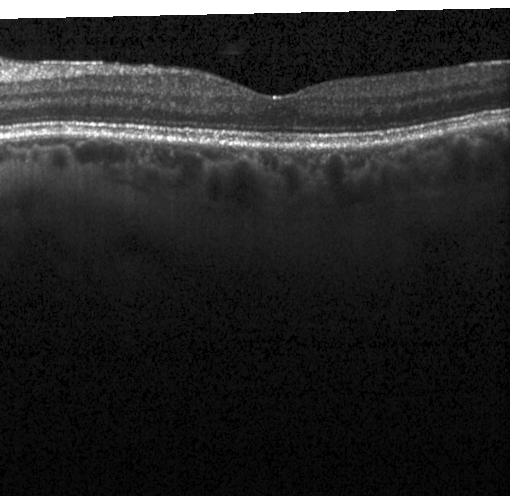

OCT B-scan; centered on the fovea; spectral-domain optical coherence tomography; Heidelberg Spectralis.
Macular OCT: no evidence of choroidal neovascularization, diabetic macular edema, or drusen.